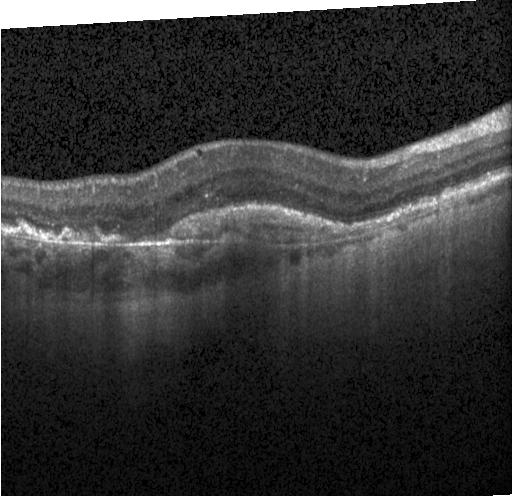
Diagnosis: choroidal neovascularization.